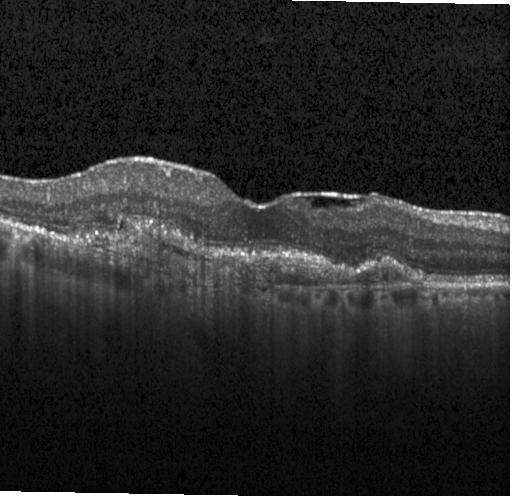 Optical coherence tomography scan. Diagnosis: CNV.